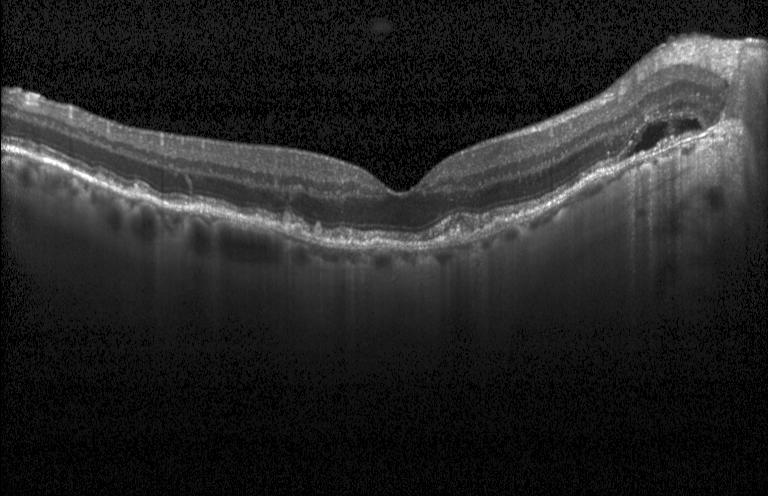

Through the macula · Heidelberg Spectralis OCT system · optical coherence tomography B-scan. Dx: a choroidal neovascular membrane.